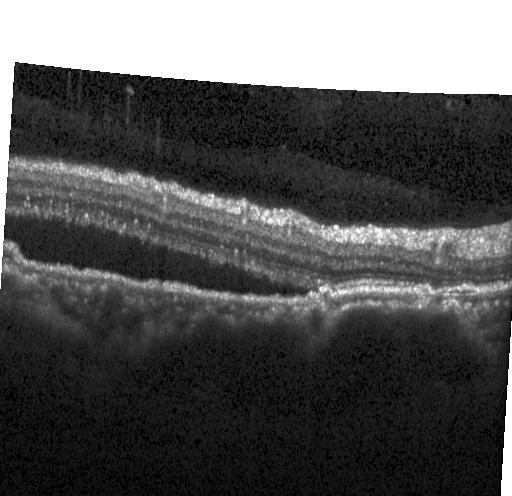
Retinal OCT B-scan — A choroidal neovascular membrane.